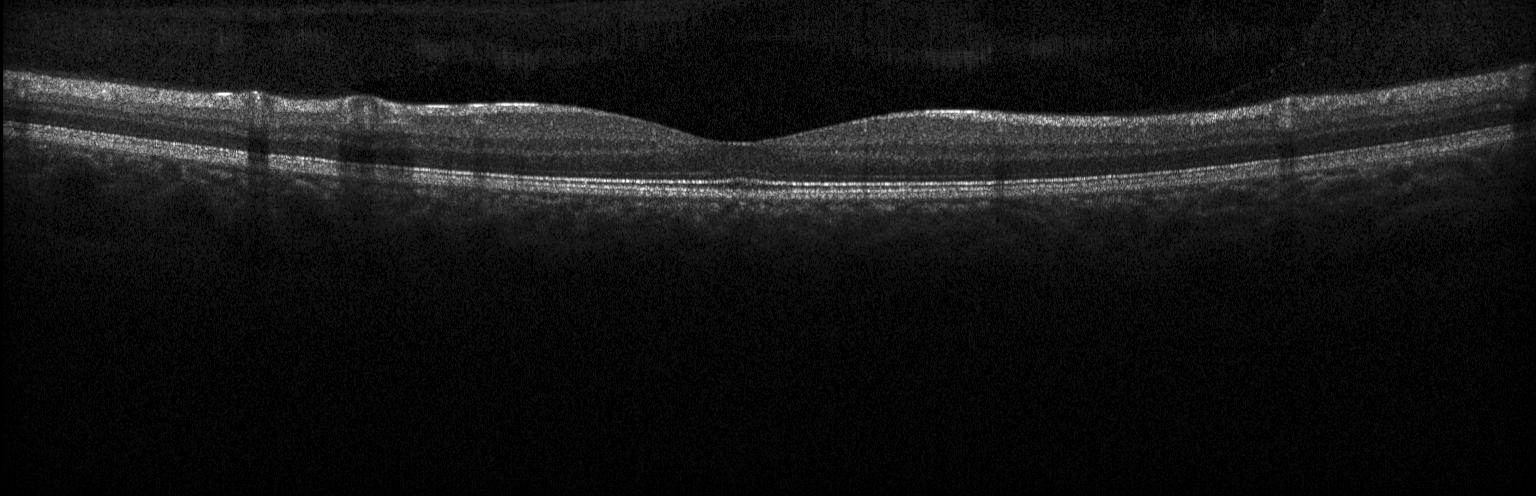
Impression: no choroidal neovascularization, no diabetic macular edema, and no drusen.